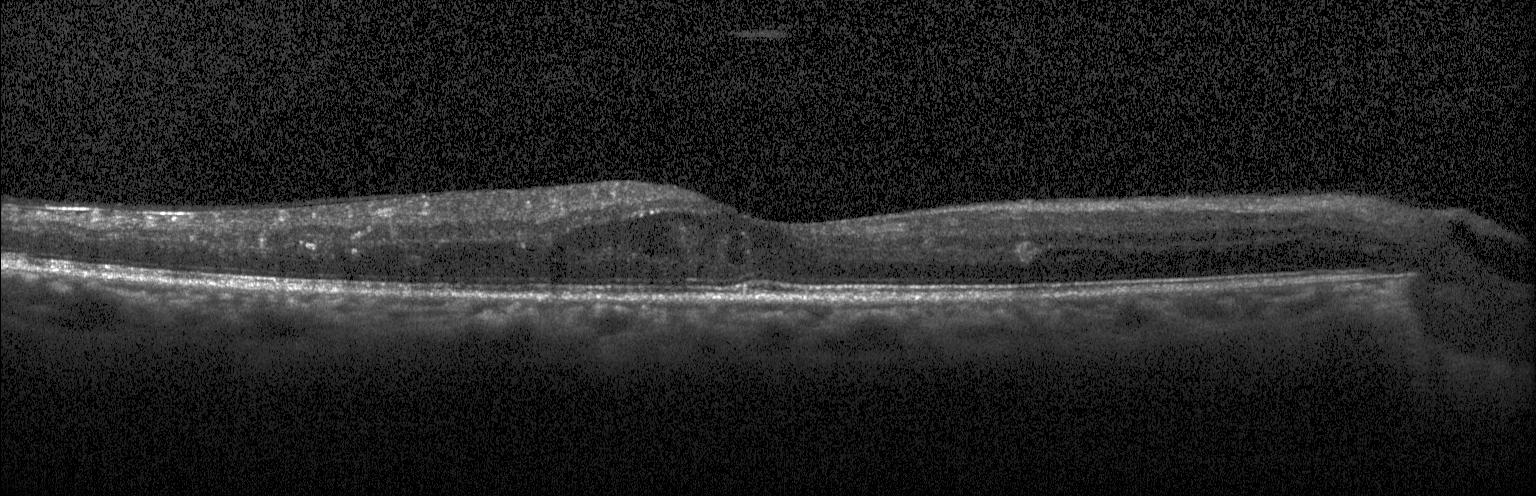 OCT B-scan. Assessment: diabetic macular edema.